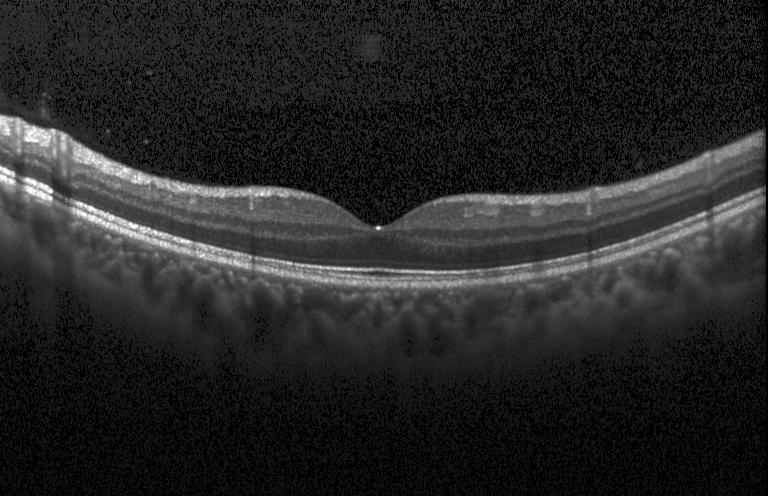

Acquired on a Heidelberg Spectralis; spectral-domain optical coherence tomography; optical coherence tomography B-scan — The scan shows neither choroidal neovascularization, diabetic macular edema, nor drusen.